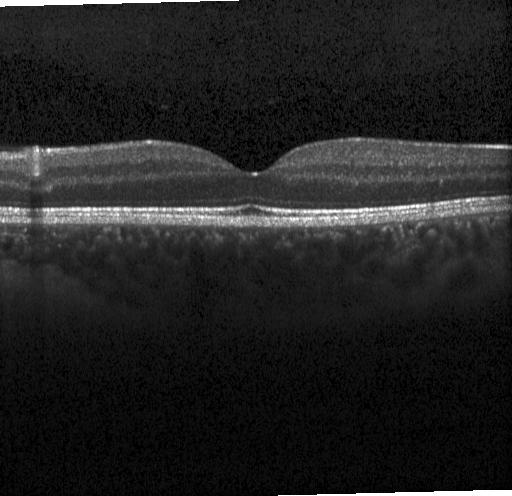

Dx: no CNV, DME, or drusen.